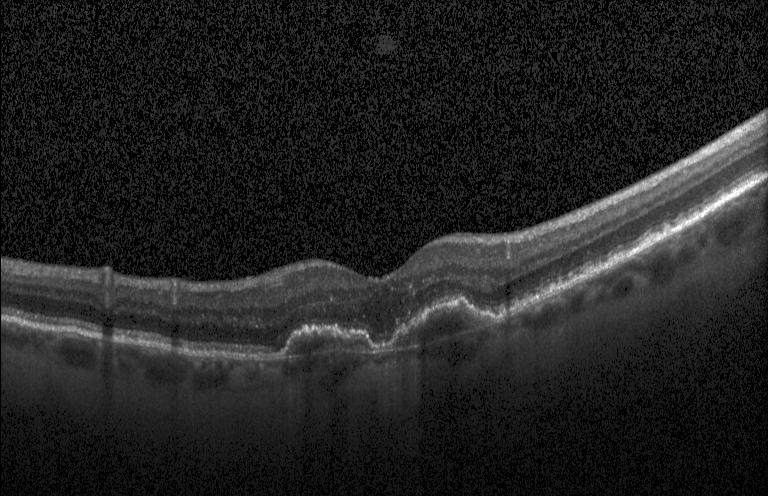

Assessment: CNV.